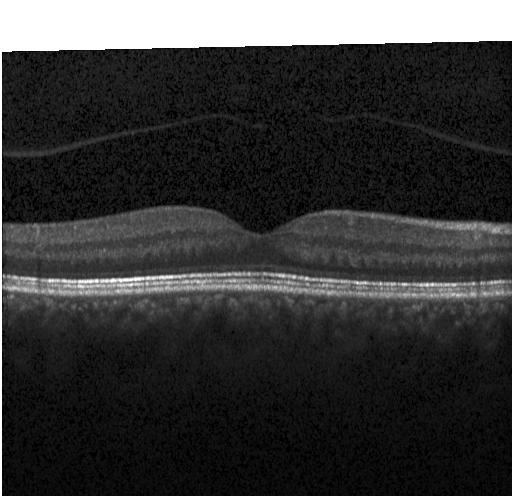

SD-OCT; retinal OCT B-scan. Macular OCT: no CNV, DME, or drusen.